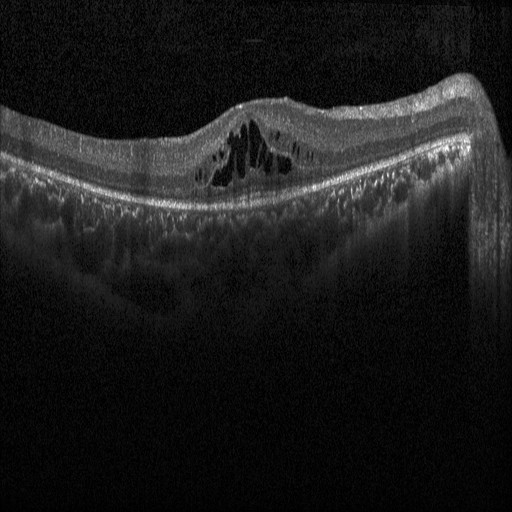
Dx: DME.